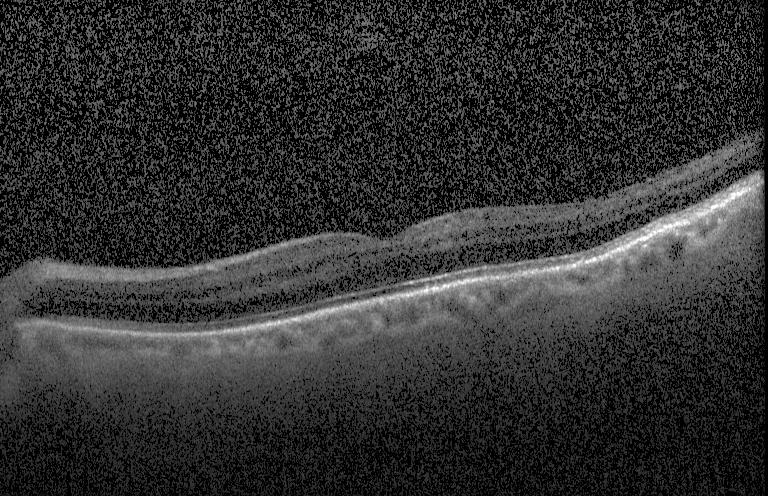 This B-scan demonstrates neither choroidal neovascularization, diabetic macular edema, nor drusen.